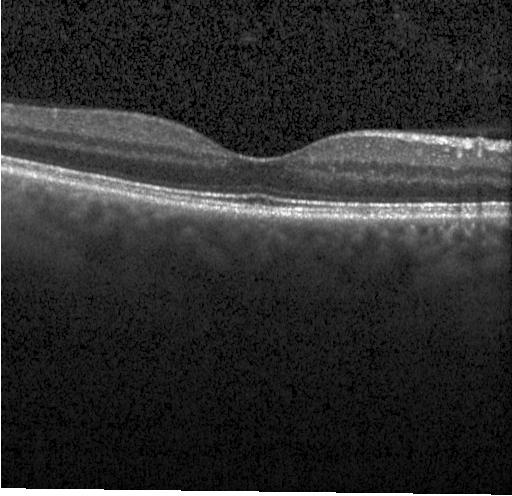 Optical coherence tomography scan. This B-scan demonstrates no choroidal neovascularization, no diabetic macular edema, and no drusen.